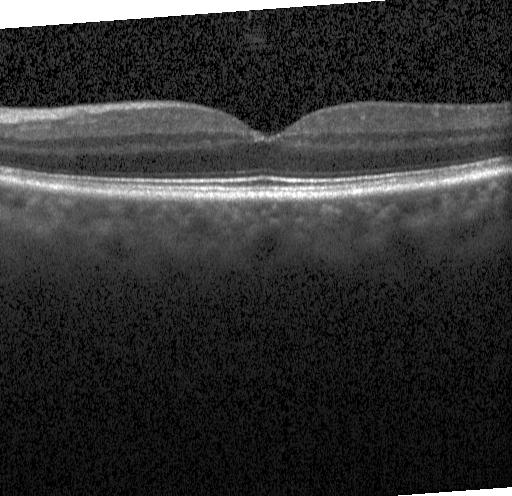

Through the macula, optical coherence tomography B-scan, Heidelberg Spectralis, spectral-domain optical coherence tomography. Neither CNV, DME, nor drusen.